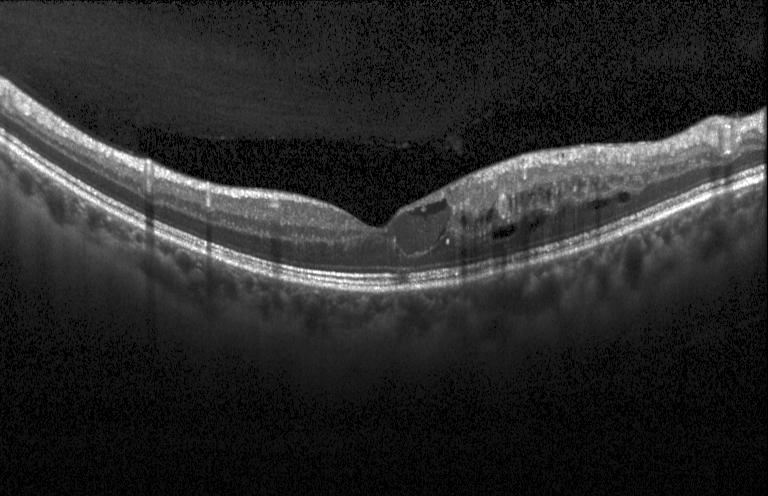 OCT B-scan showing DME.